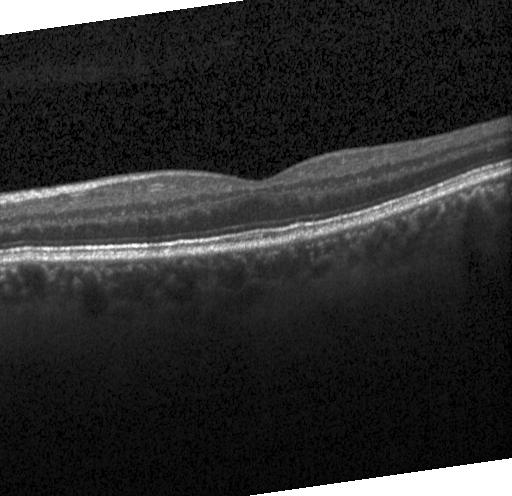 Spectral-domain OCT; Heidelberg Spectralis; retinal OCT B-scan
OCT finding: no choroidal neovascularization, no diabetic macular edema, and no drusen.